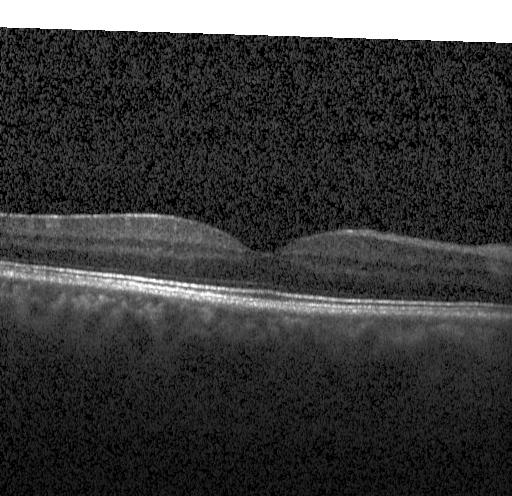

Retinal OCT B-scan. Spectral-domain optical coherence tomography. Impression: no choroidal neovascularization, diabetic macular edema, or drusen.